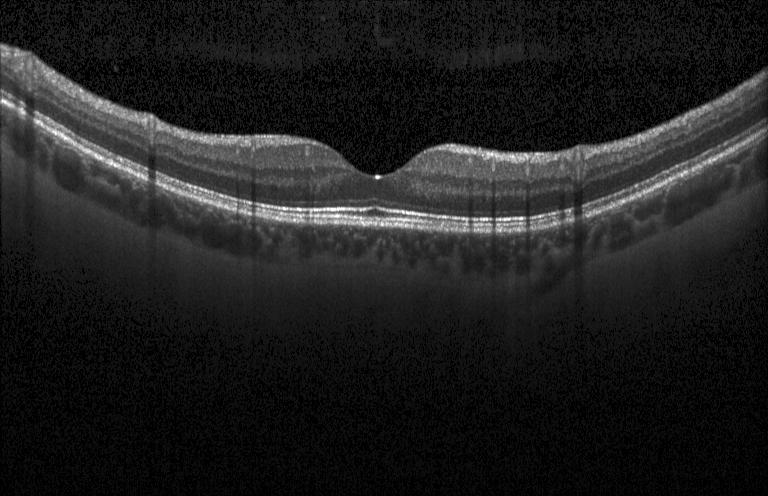
Retinal OCT cross-section. Horizontal scan through the fovea. Heidelberg Spectralis OCT system — This B-scan demonstrates no CNV, DME, or drusen.